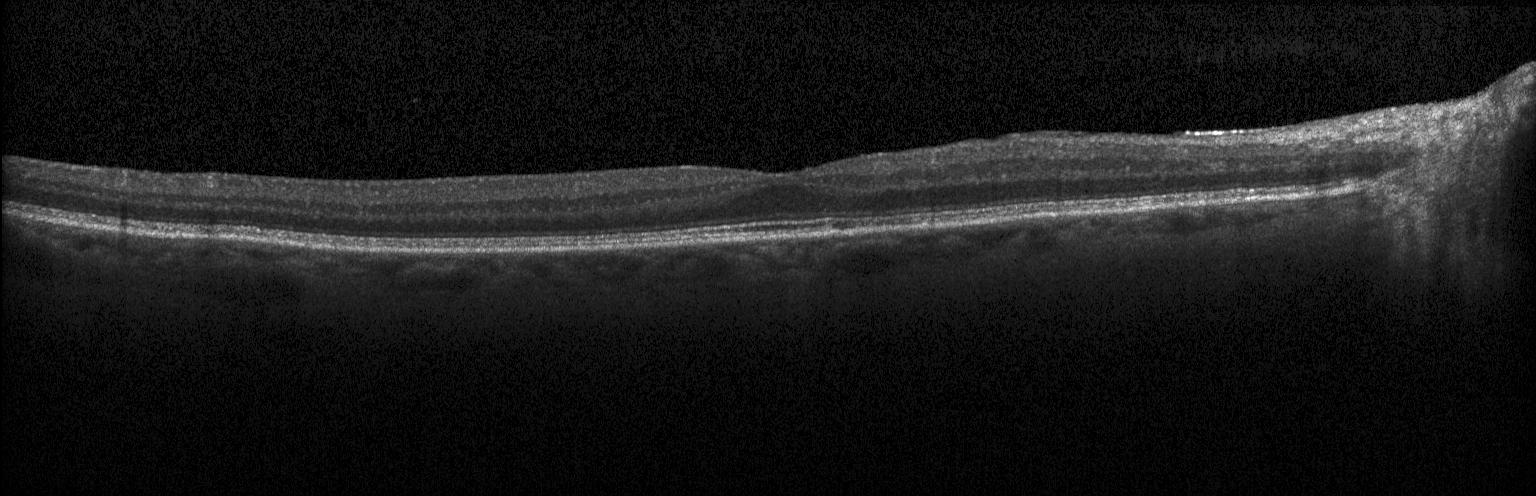 Assessment: neither choroidal neovascularization, diabetic macular edema, nor drusen.